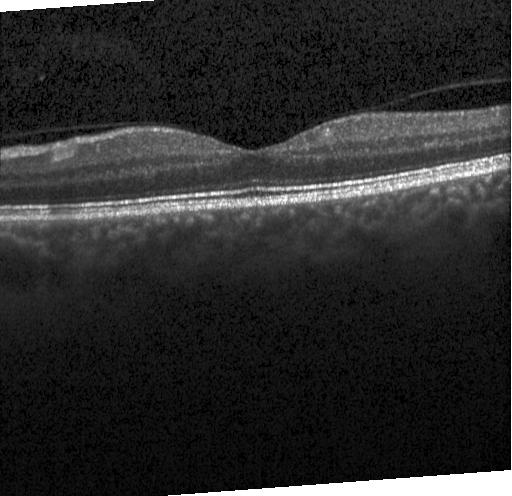 Impression: no choroidal neovascularization, diabetic macular edema, or drusen.